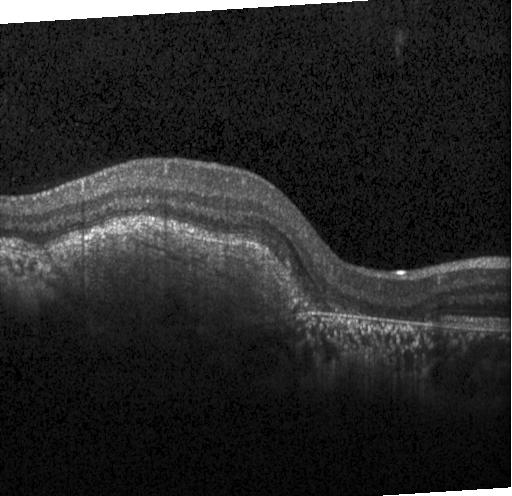 Optical coherence tomography B-scan — Macular OCT: a choroidal neovascular membrane.